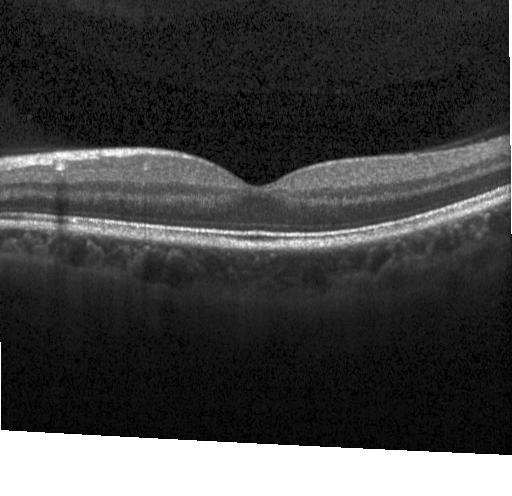
Diagnosis: no choroidal neovascularization, diabetic macular edema, or drusen.